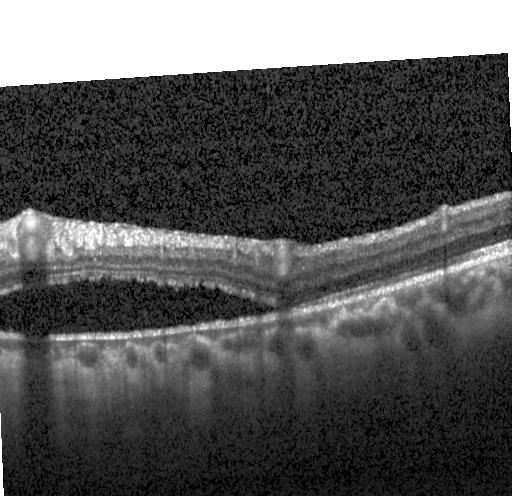 Diagnosis: a choroidal neovascular membrane.